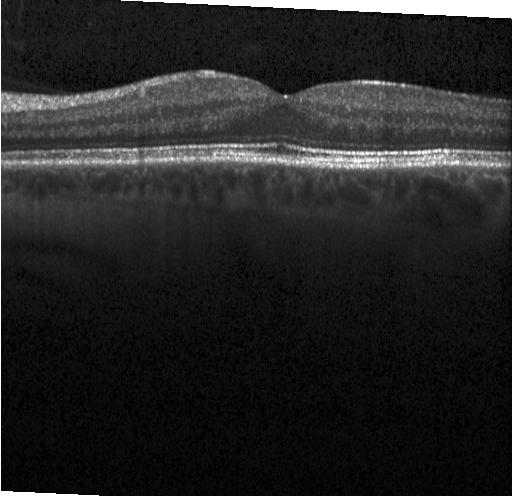
Assessment: no evidence of choroidal neovascularization, diabetic macular edema, or drusen.